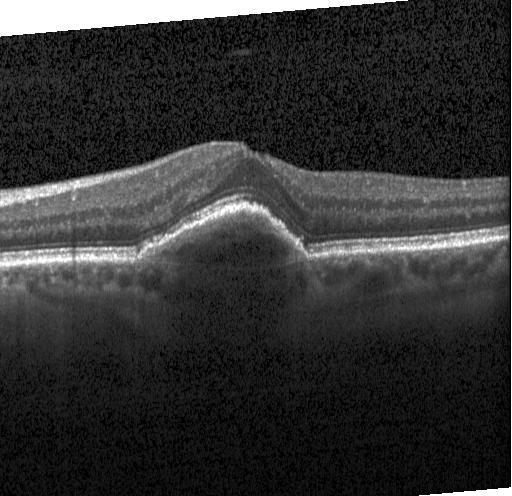 Finding: a choroidal neovascular membrane.